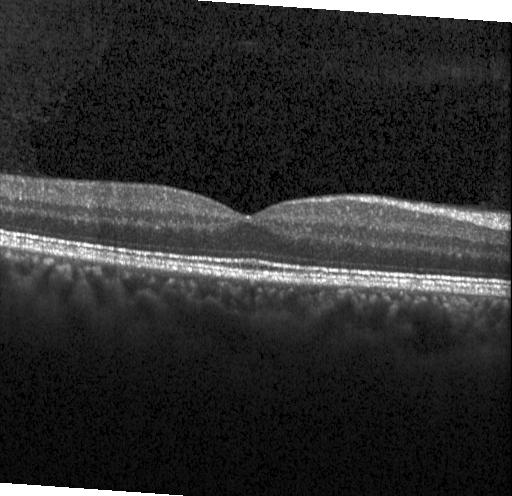

Macular scan; spectral-domain optical coherence tomography; Heidelberg Spectralis OCT system; optical coherence tomography scan
No choroidal neovascularization, diabetic macular edema, or drusen.